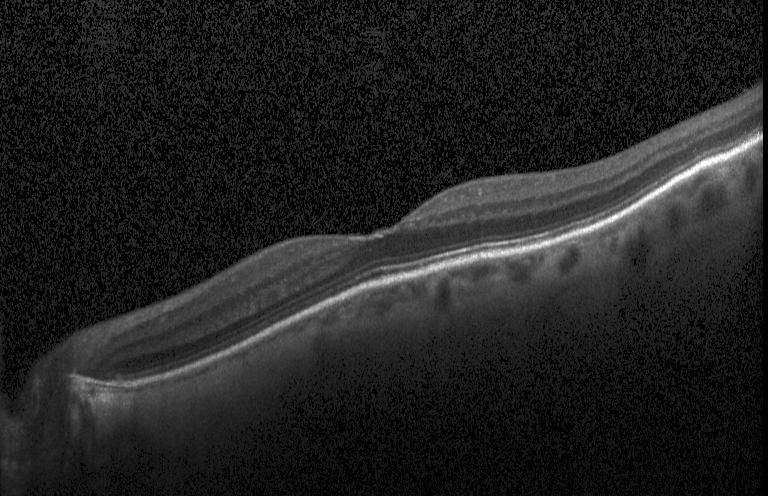
Retinal OCT B-scan; SD-OCT; Heidelberg Spectralis; through the macula.
This B-scan demonstrates no evidence of CNV, DME, or drusen.